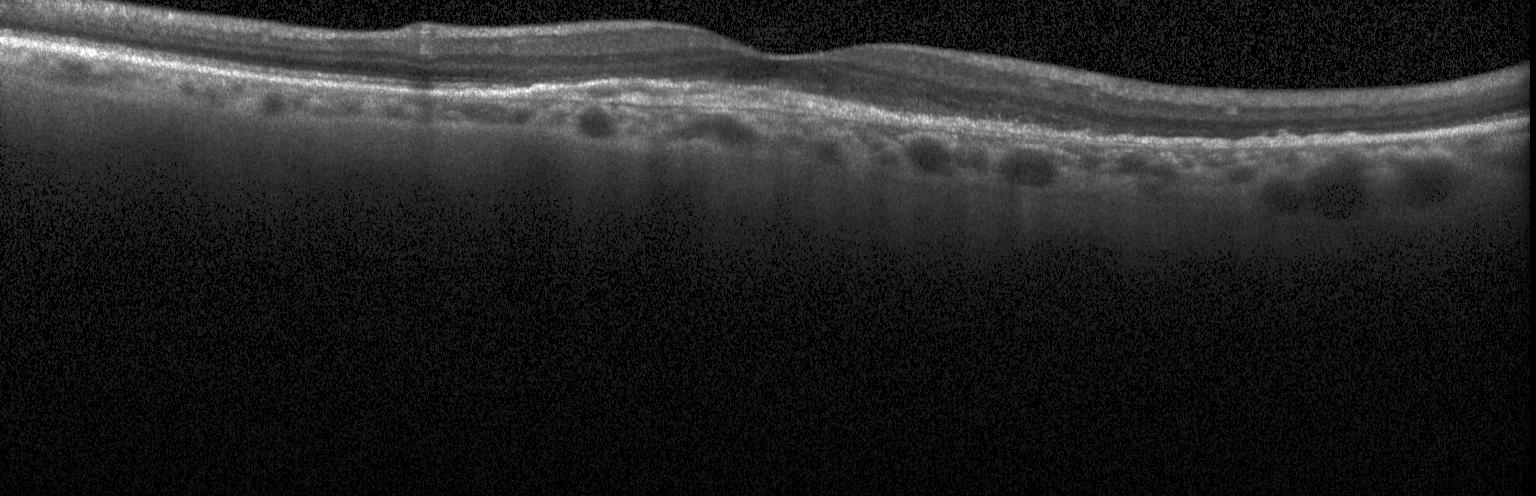
Acquired on a Heidelberg Spectralis, retinal OCT cross-section — Finding: choroidal neovascularization (CNV).